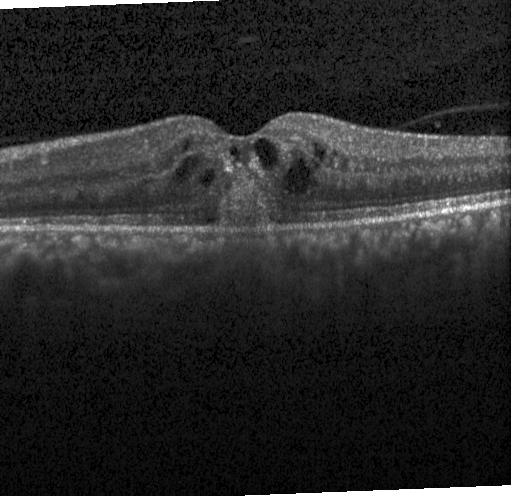
Optical coherence tomography scan, spectral-domain optical coherence tomography — The scan shows a choroidal neovascular membrane.